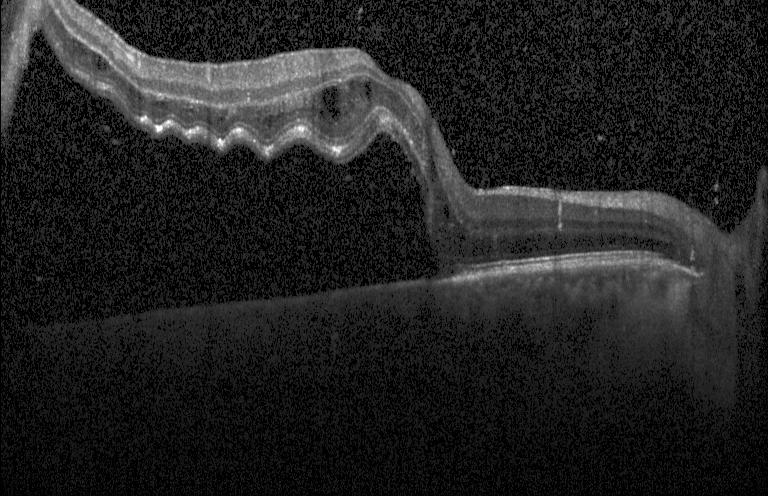

Instrument: Heidelberg Spectralis, SD-OCT, OCT B-scan, macular scan — Assessment: DME.